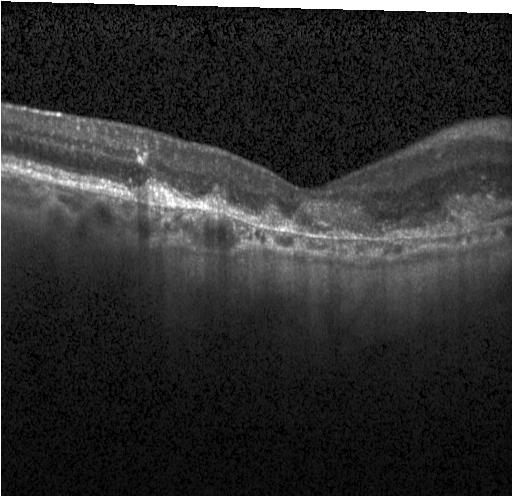 Diagnosis: CNV.